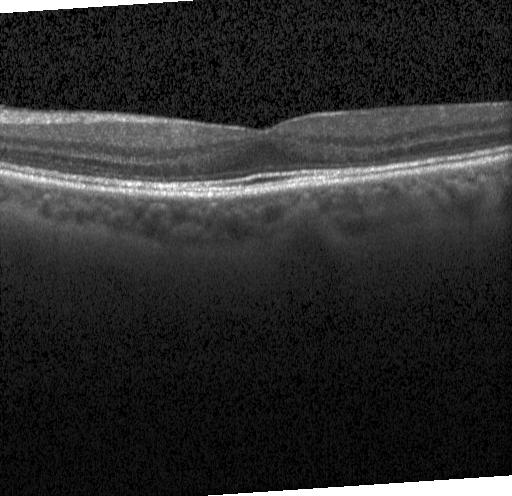 Horizontal scan through the fovea, Heidelberg Spectralis OCT system, spectral-domain optical coherence tomography, retinal OCT B-scan.
Impression: no CNV, DME, or drusen.